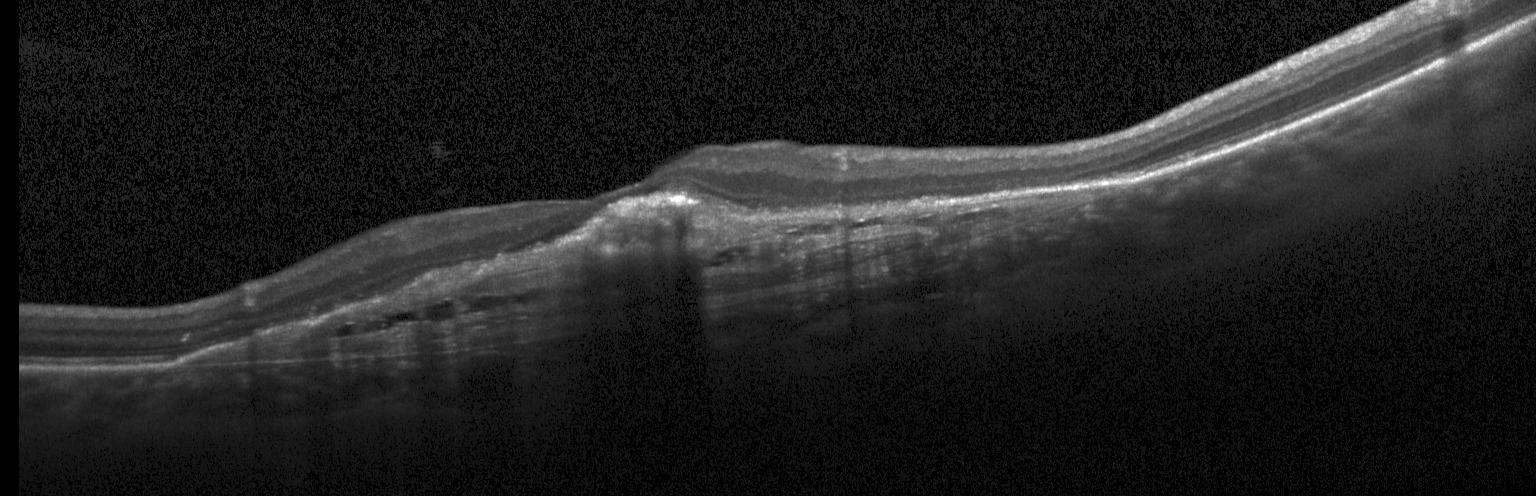 Spectral-domain optical coherence tomography, Heidelberg Spectralis OCT system, OCT line scan, centered on the fovea
Finding: choroidal neovascularization (CNV).